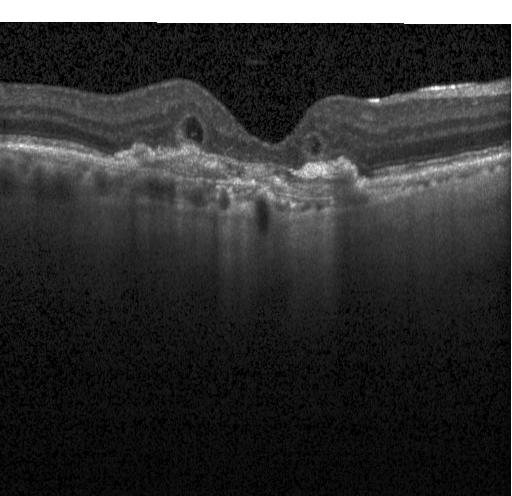 Macular scan, spectral-domain optical coherence tomography, optical coherence tomography B-scan — Finding: CNV.